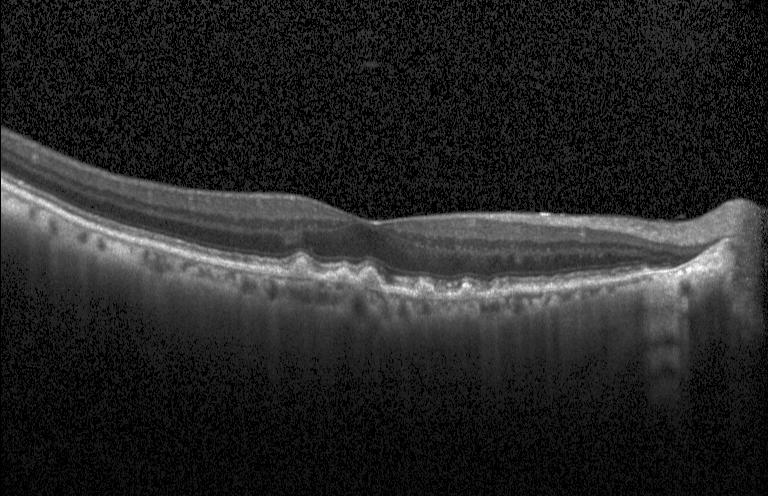

SD-OCT · through the macula · optical coherence tomography scan · Heidelberg Spectralis. Impression: sub-RPE drusenoid deposits.